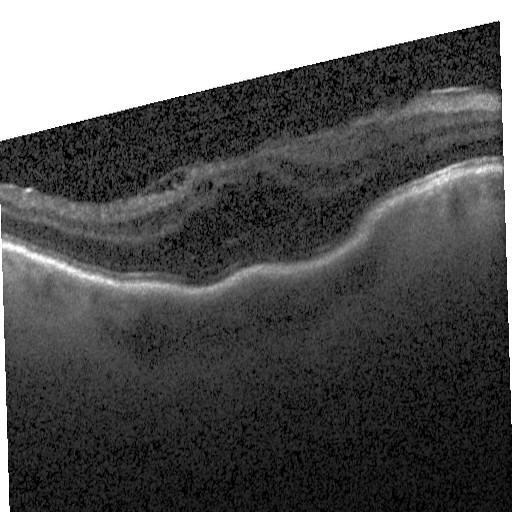
Instrument: Heidelberg Spectralis. Horizontal scan through the fovea. Retinal OCT cross-section. Spectral-domain optical coherence tomography. This B-scan demonstrates DME.